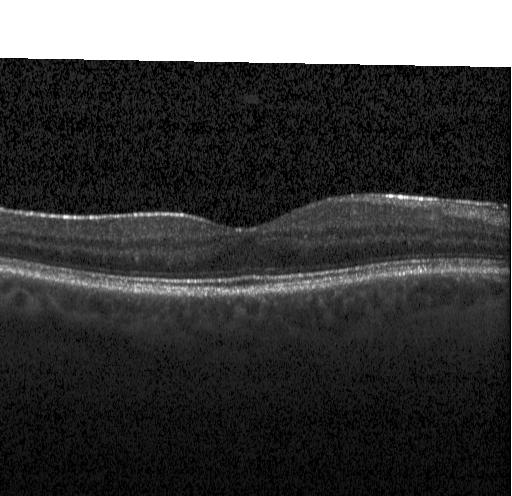

Acquired on a Heidelberg Spectralis · horizontal scan through the fovea · retinal OCT B-scan. Macular OCT: neither choroidal neovascularization, diabetic macular edema, nor drusen.